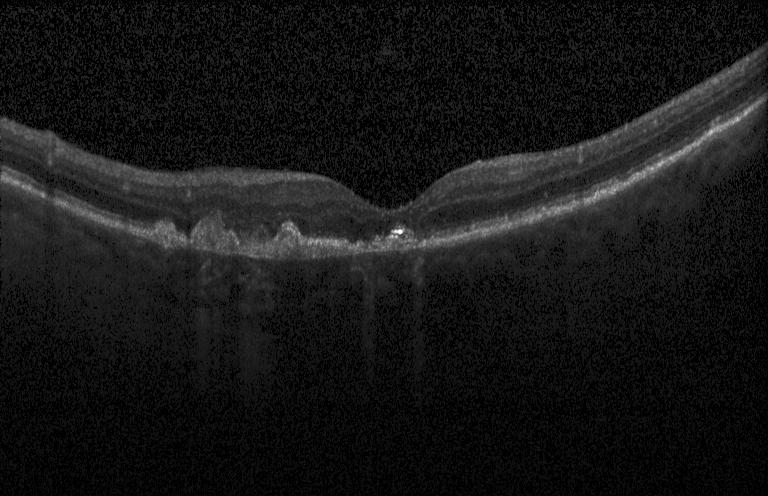 Retinal OCT cross-section — Assessment: a choroidal neovascular membrane.